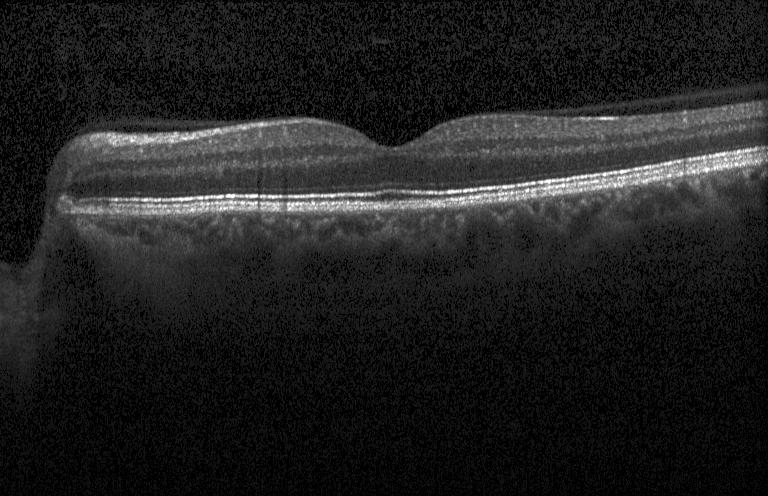
Diagnosis: no choroidal neovascularization, no diabetic macular edema, and no drusen.